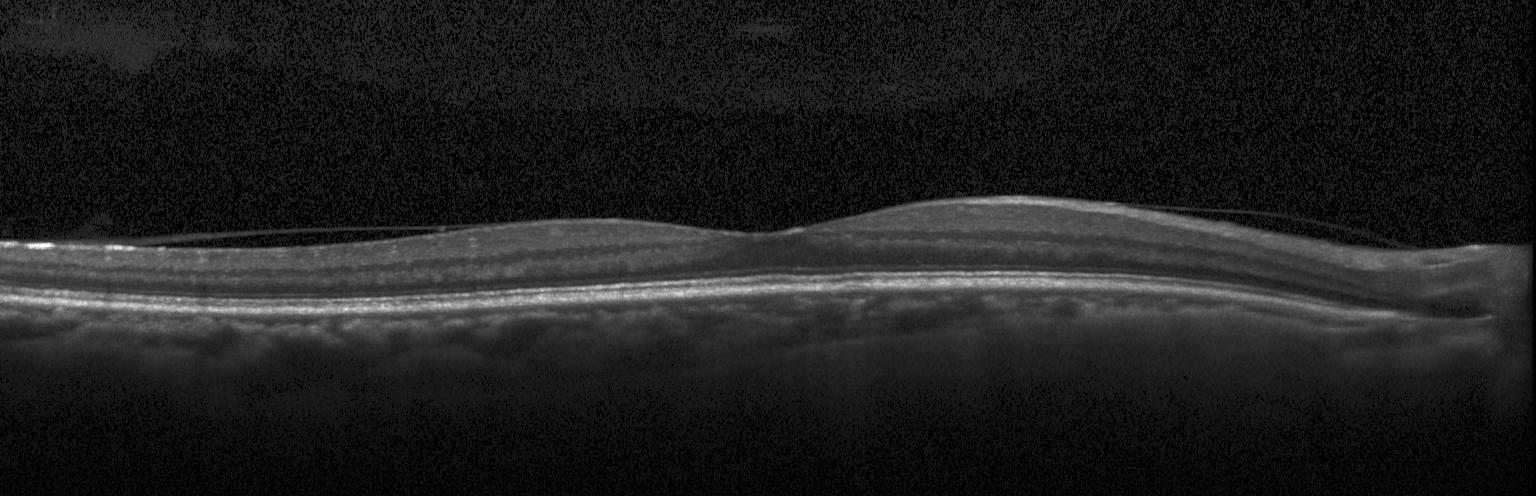 Neither choroidal neovascularization, diabetic macular edema, nor drusen.